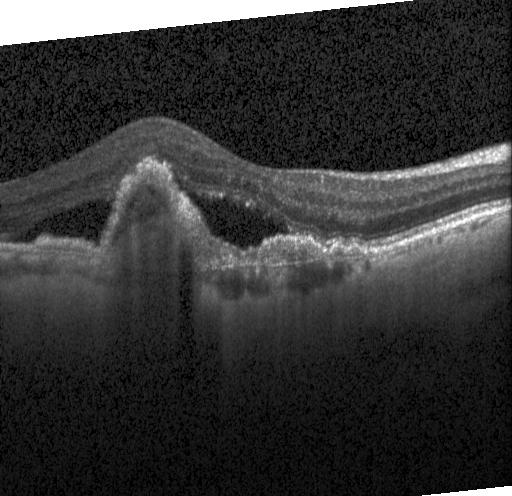
Spectral-domain OCT B-scan: a choroidal neovascular membrane.